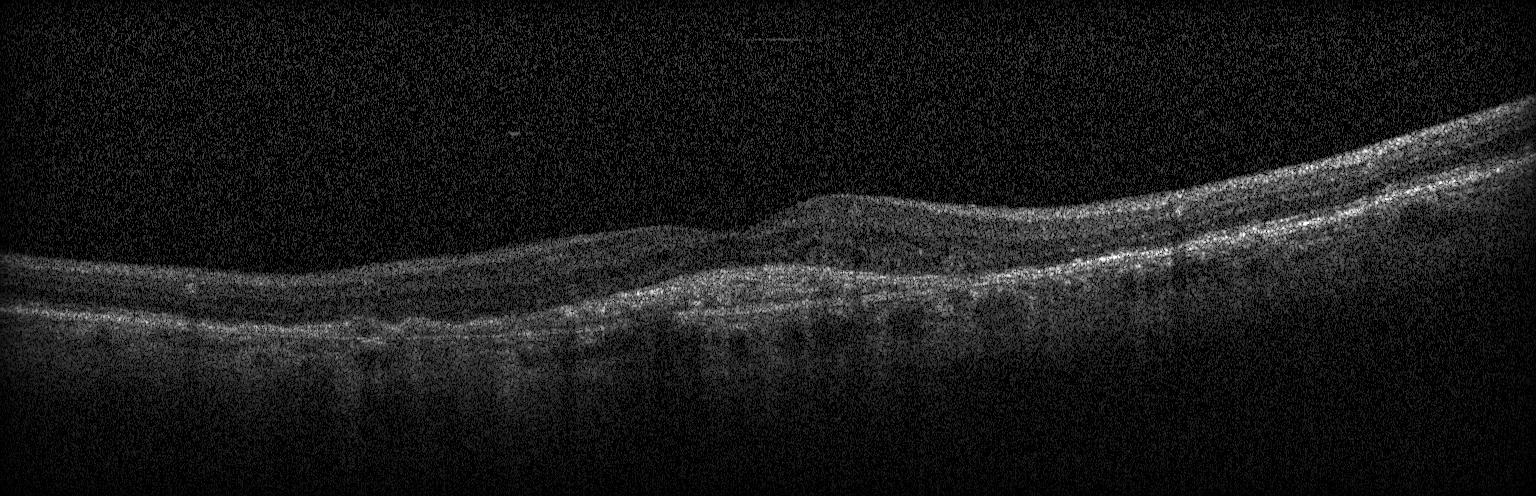 Spectral-domain OCT, through the macula, instrument: Heidelberg Spectralis, OCT line scan — Diagnosis: a choroidal neovascular membrane.